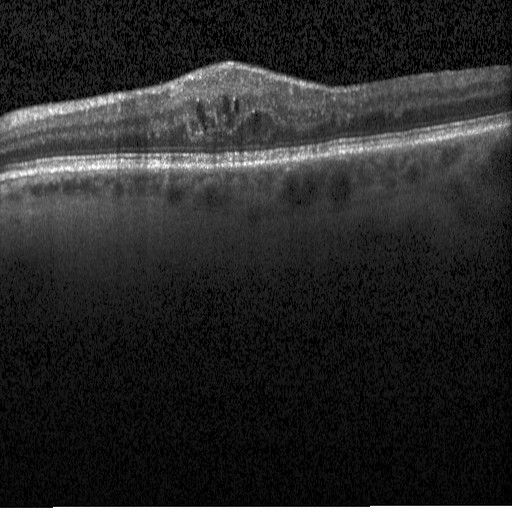
Retinal OCT B-scan. Spectral-domain optical coherence tomography. Fovea-centered. Heidelberg Spectralis. Dx: diabetic macular edema (DME).